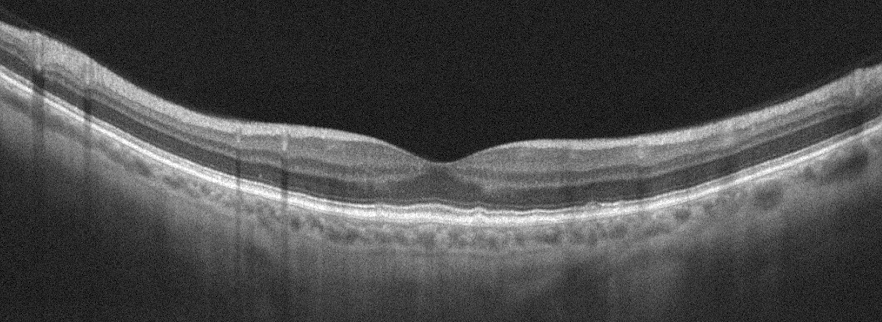 Optical coherence tomography B-scan. Left eye. Macular scan — Finding: AMD.